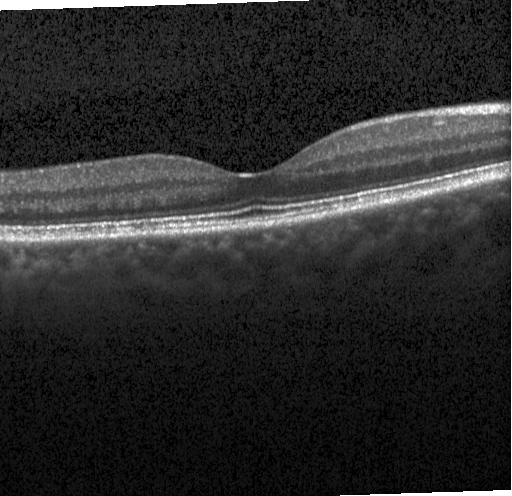

No choroidal neovascularization, diabetic macular edema, or drusen.